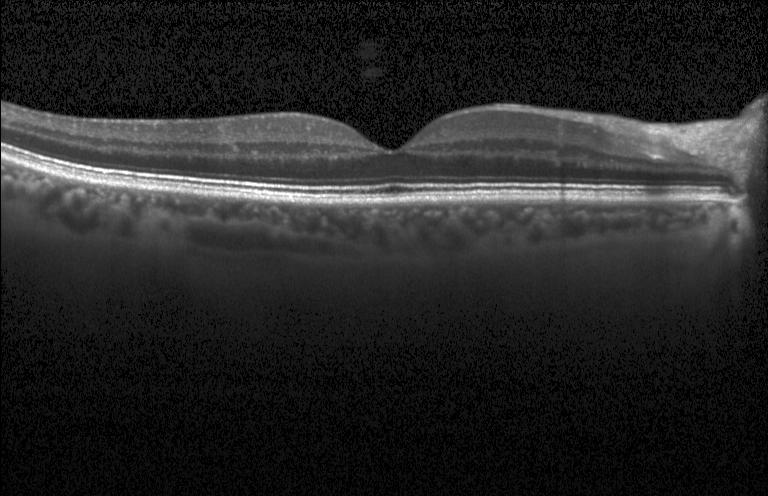

This B-scan demonstrates neither choroidal neovascularization, diabetic macular edema, nor drusen.